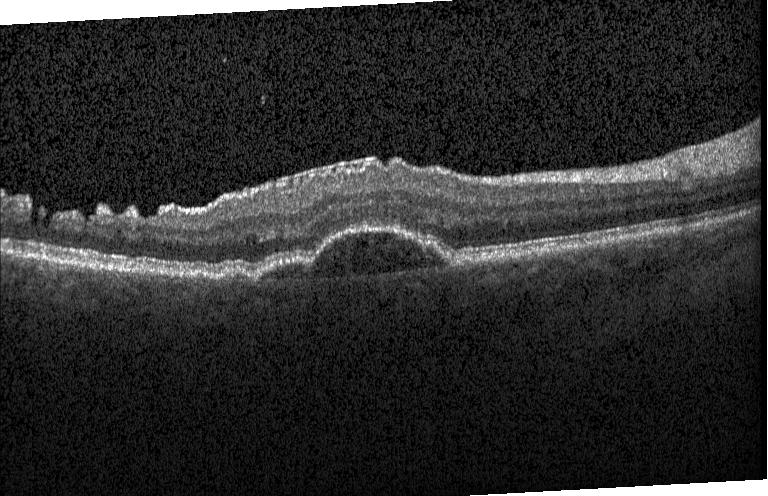 Retinal OCT cross-section. Instrument: Heidelberg Spectralis. Centered on the fovea. Spectral-domain OCT. This B-scan demonstrates choroidal neovascularization (CNV).